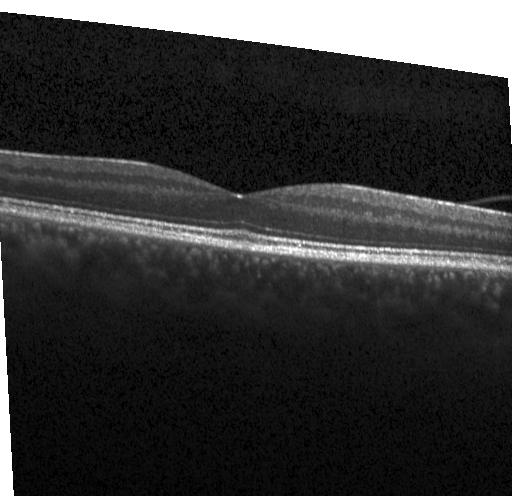

Macular OCT demonstrating neither choroidal neovascularization, diabetic macular edema, nor drusen.